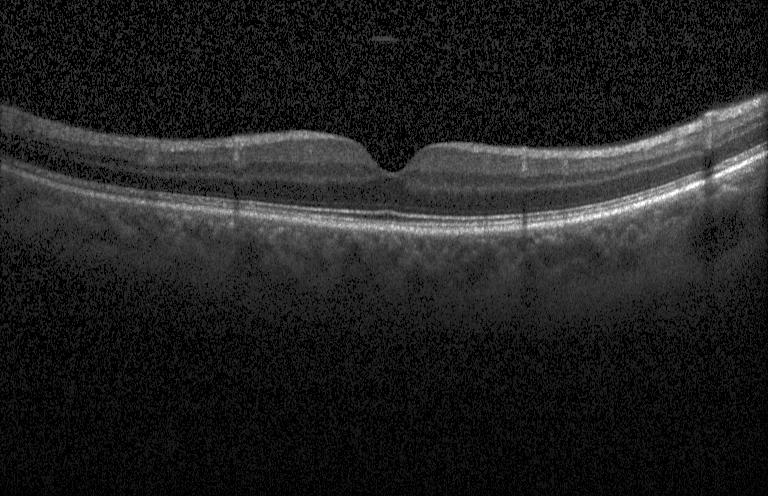
Finding: neither CNV, DME, nor drusen.